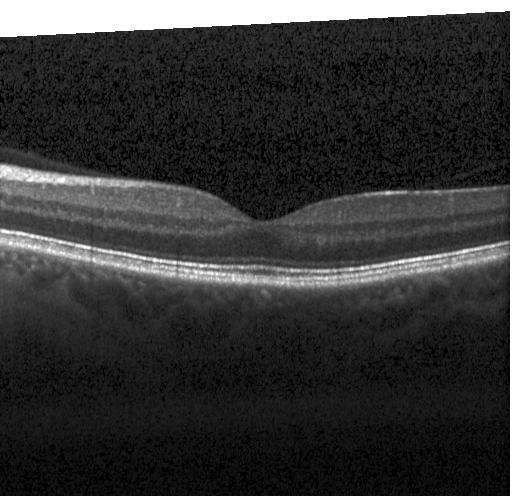

This B-scan demonstrates no choroidal neovascularization, diabetic macular edema, or drusen.